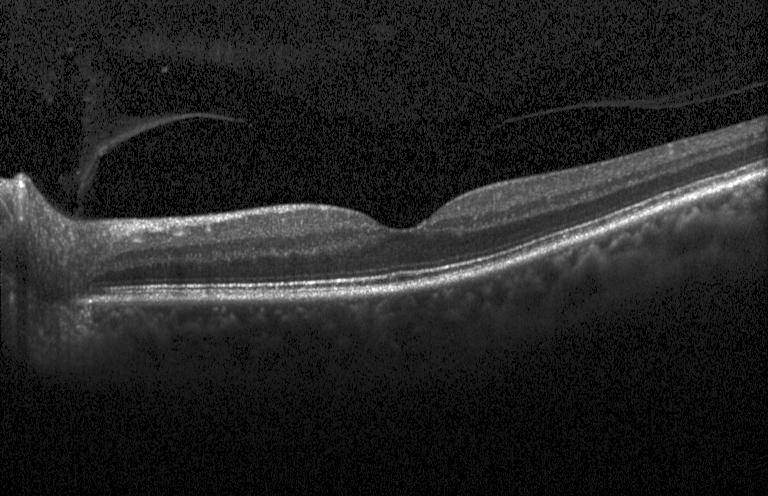 Spectral-domain optical coherence tomography. Acquired on a Heidelberg Spectralis. OCT B-scan. Through the macula
This B-scan demonstrates no CNV, DME, or drusen.